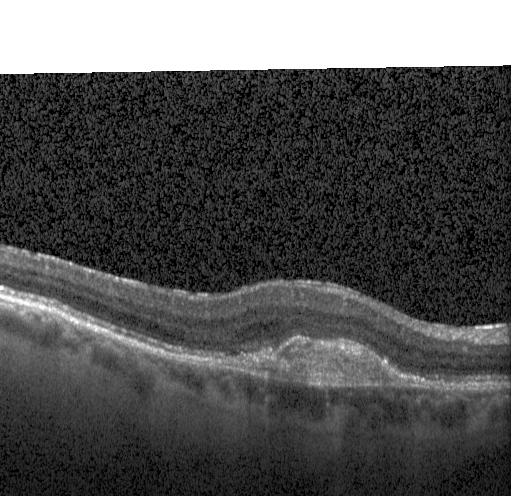

Heidelberg Spectralis. Optical coherence tomography B-scan. Macular scan. Spectral-domain optical coherence tomography — Diagnosis: choroidal neovascularization.